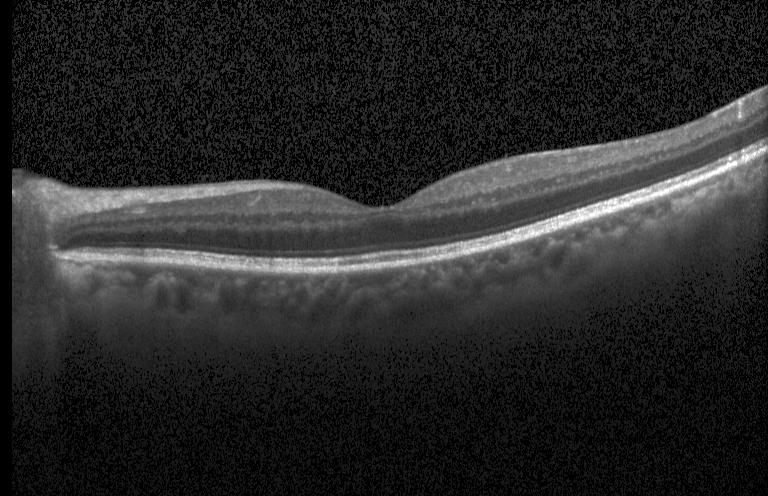
This B-scan demonstrates no choroidal neovascularization, no diabetic macular edema, and no drusen.